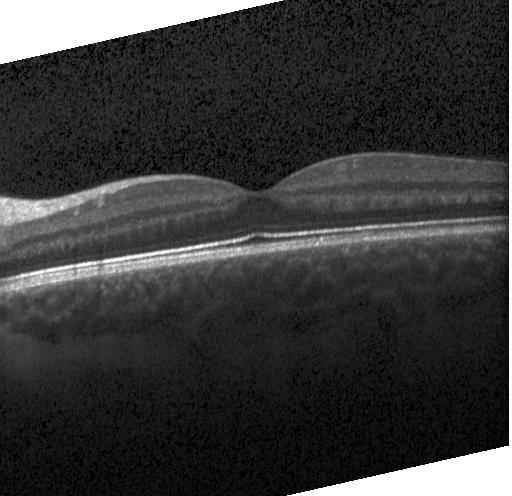 Optical coherence tomography scan, SD-OCT
Neither CNV, DME, nor drusen.